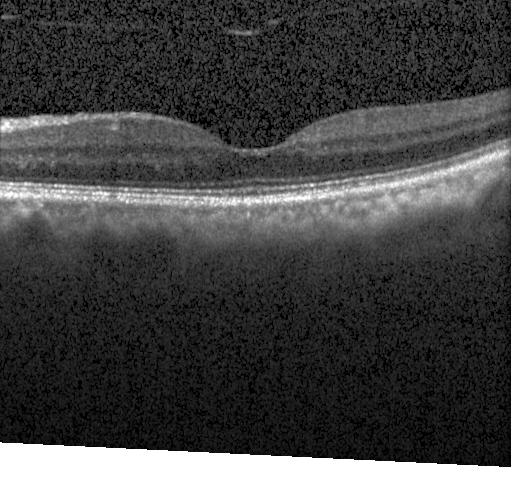

Heidelberg Spectralis OCT system; retinal OCT cross-section. This B-scan demonstrates no CNV, no DME, and no drusen.